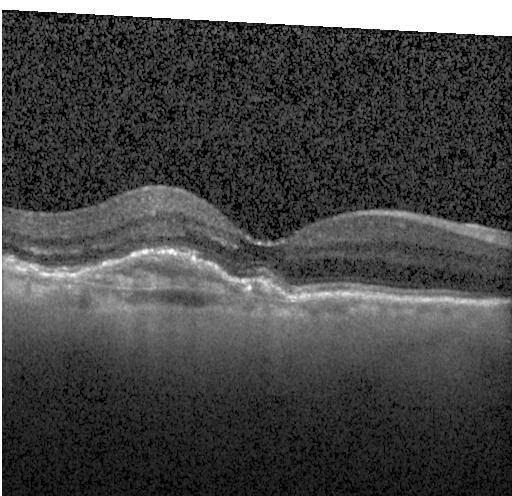

Through the macula, OCT line scan, SD-OCT
Diagnosis: a choroidal neovascular membrane.